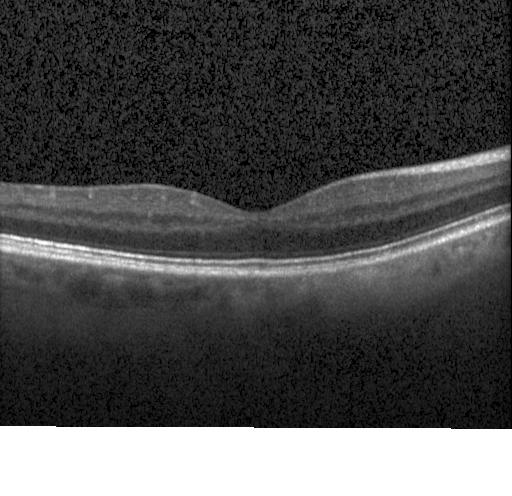 Retinal OCT B-scan. Spectral-domain OCT. No choroidal neovascularization, no diabetic macular edema, and no drusen.